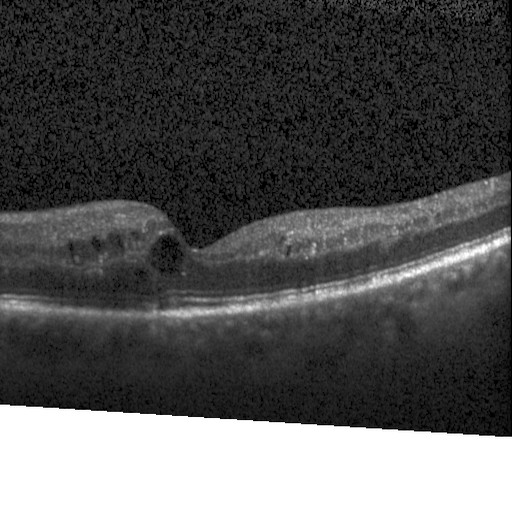 Centered on the fovea; instrument: Heidelberg Spectralis; spectral-domain OCT; optical coherence tomography B-scan
Finding: DME.